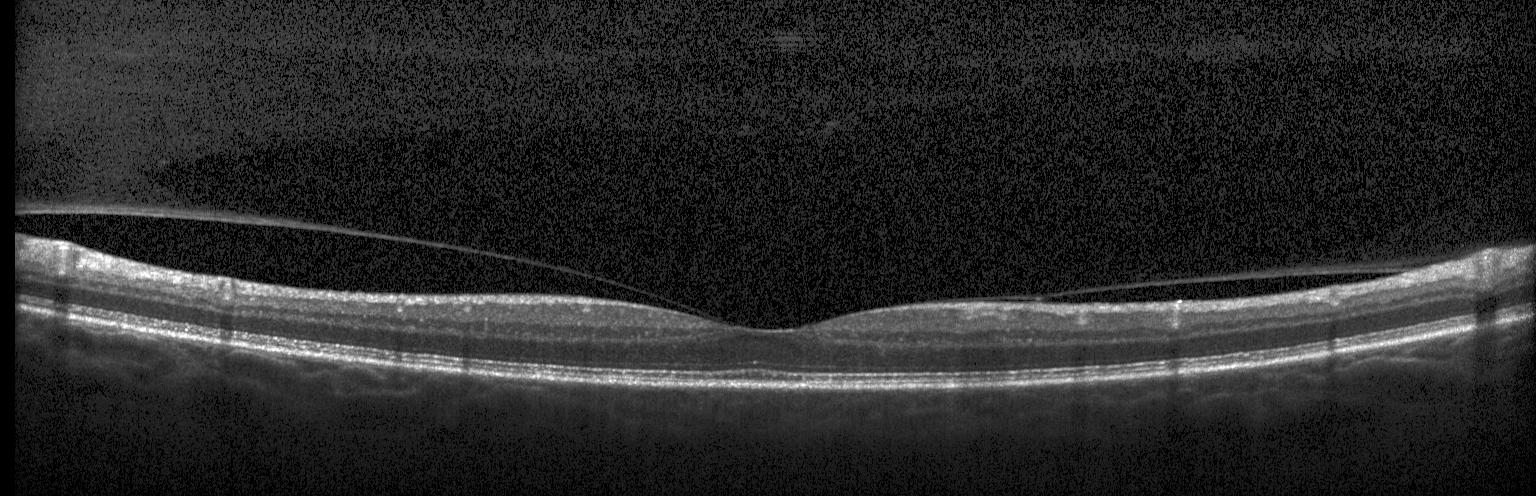 Fovea-centered; SD-OCT; retinal OCT cross-section — Finding: no CNV, no DME, and no drusen.